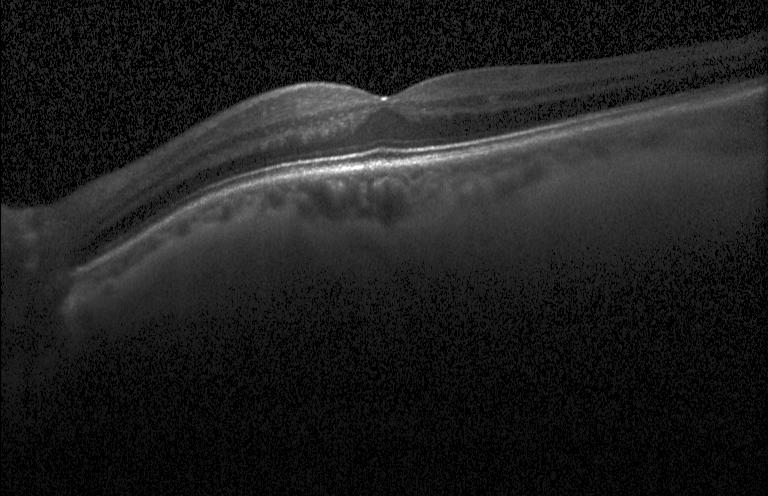 Optical coherence tomography B-scan. Spectral-domain OCT — Impression: no choroidal neovascularization, diabetic macular edema, or drusen.